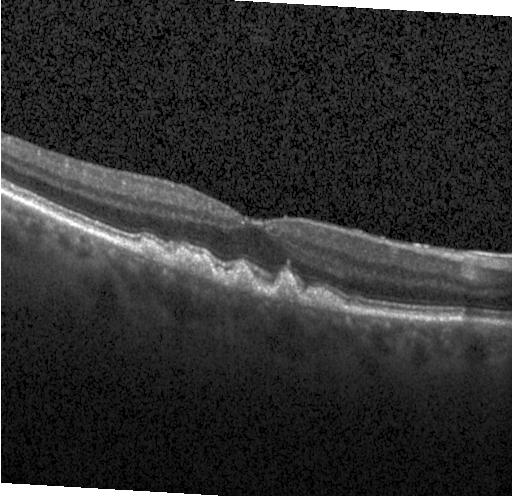

OCT finding: multiple drusen.